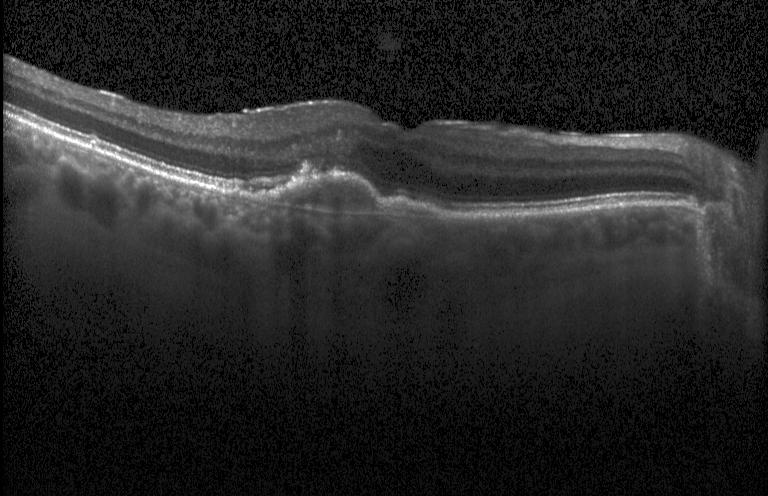
Optical coherence tomography scan. This B-scan demonstrates a choroidal neovascular membrane.